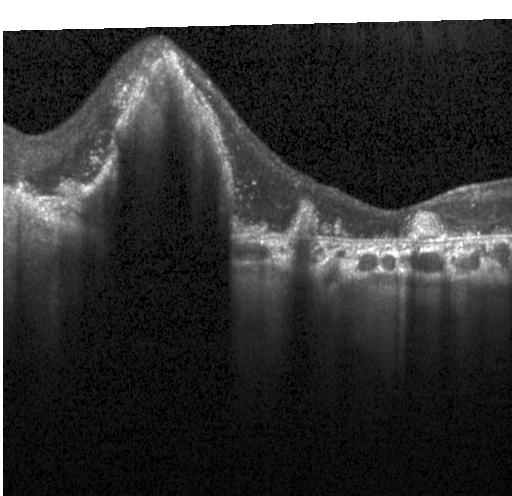
Assessment: a choroidal neovascular membrane.